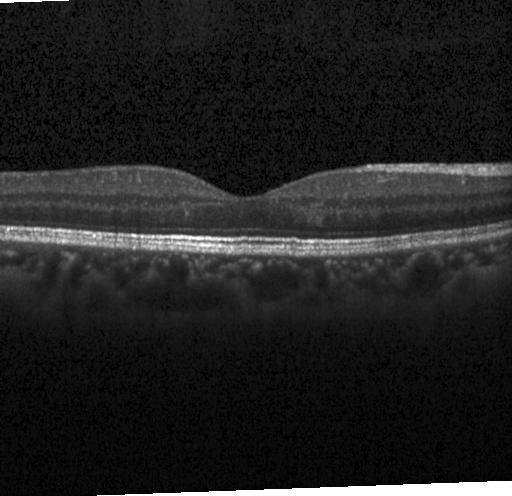
Instrument: Heidelberg Spectralis, spectral-domain optical coherence tomography, OCT line scan, through the macula — Diagnosis: no CNV, no DME, and no drusen.